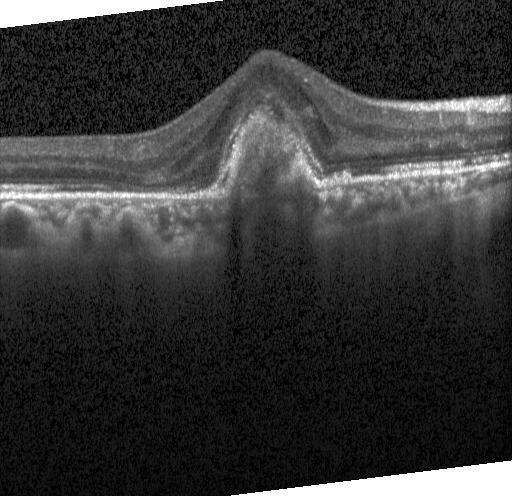

OCT line scan
OCT finding: CNV.